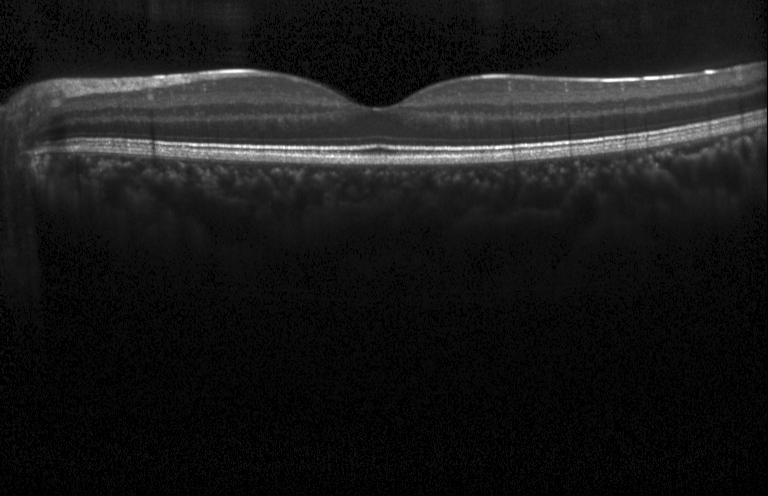 OCT scan showing no evidence of choroidal neovascularization, diabetic macular edema, or drusen.